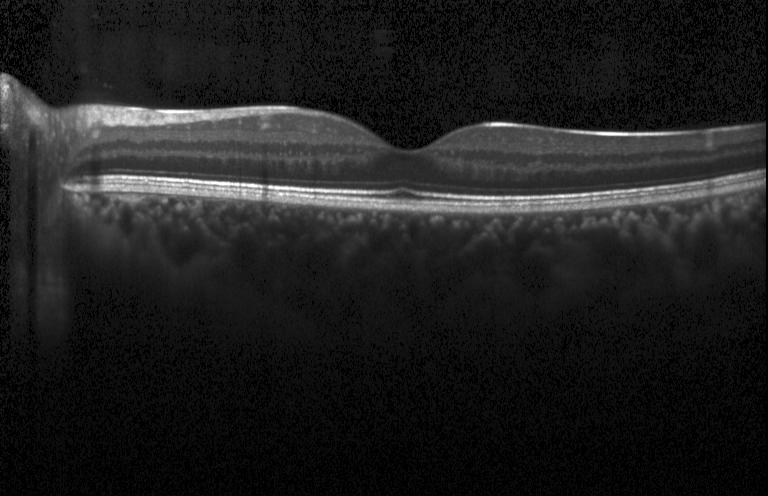

OCT line scan; Heidelberg Spectralis
Finding: neither CNV, DME, nor drusen.